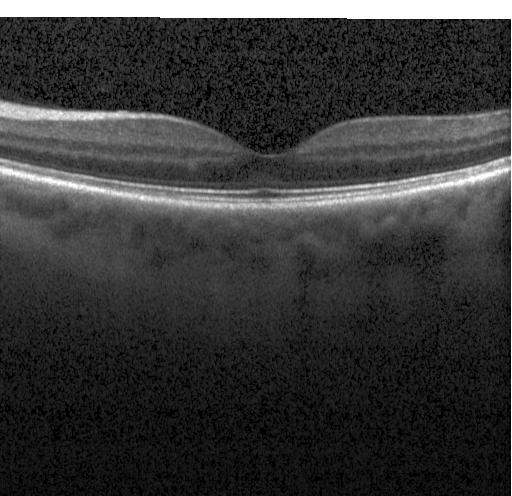
Optical coherence tomography B-scan, spectral-domain optical coherence tomography, Heidelberg Spectralis
OCT finding: neither choroidal neovascularization, diabetic macular edema, nor drusen.